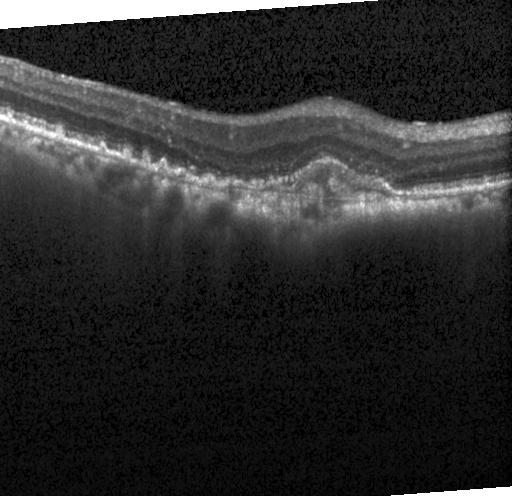

OCT finding: a choroidal neovascular membrane.